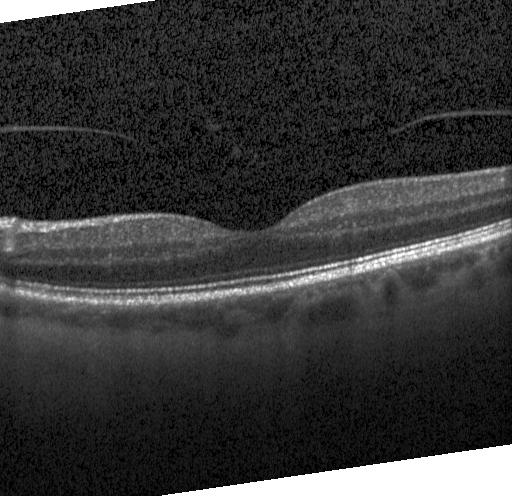
Spectral-domain OCT · retinal OCT B-scan · centered on the fovea · Heidelberg Spectralis OCT system. Finding: neither CNV, DME, nor drusen.